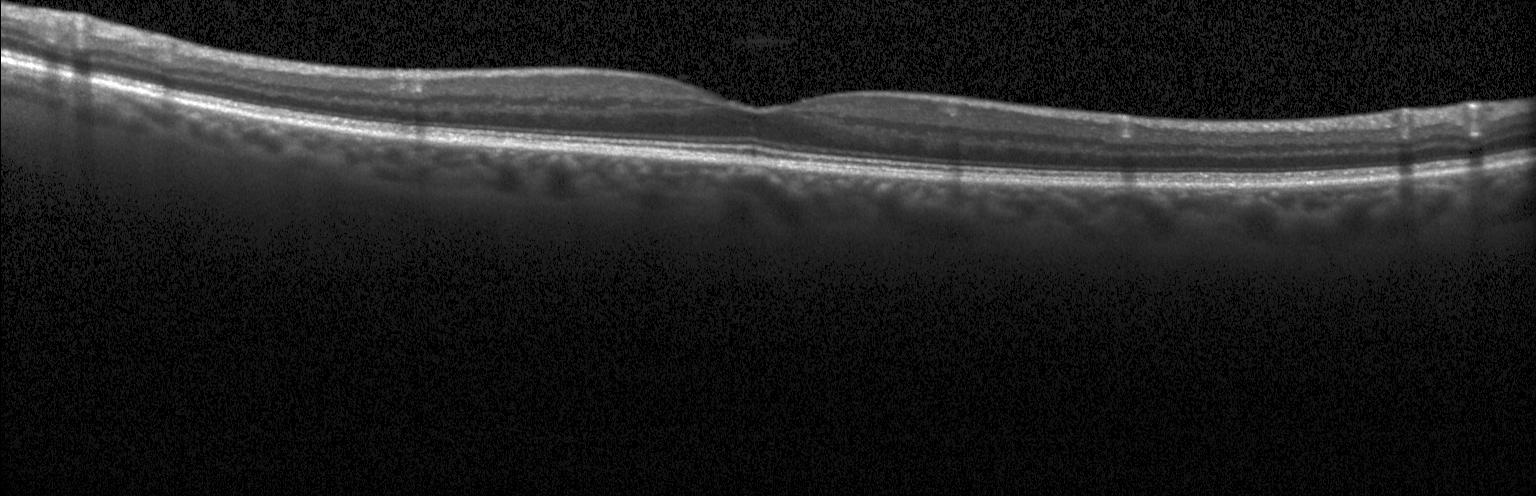

OCT B-scan; acquired on a Heidelberg Spectralis; macular scan — This B-scan demonstrates no choroidal neovascularization, no diabetic macular edema, and no drusen.